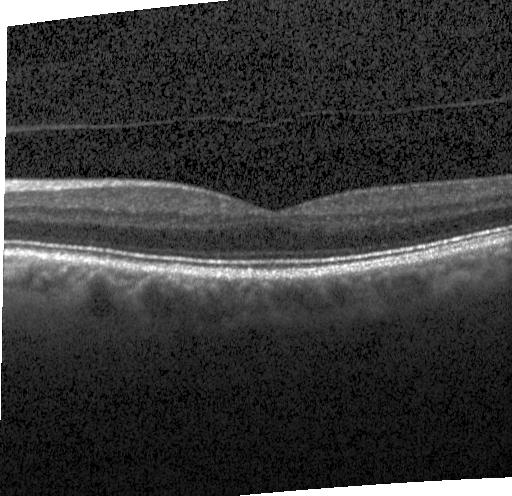 OCT B-scan showing no CNV, no DME, and no drusen.